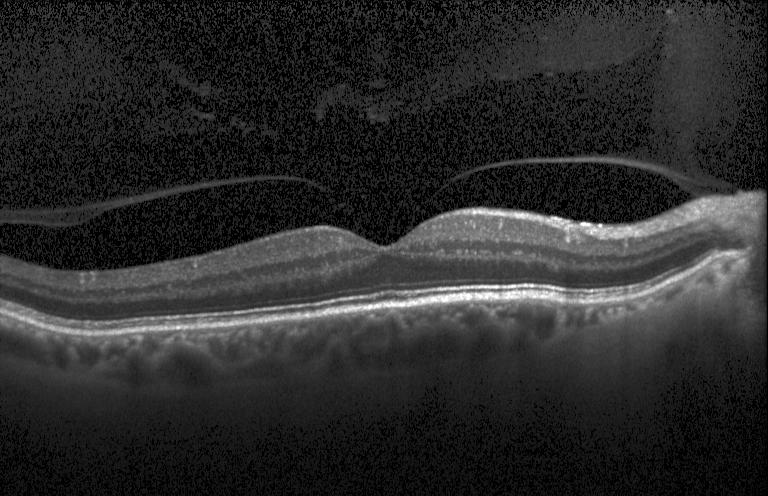 Macular OCT: no evidence of choroidal neovascularization, diabetic macular edema, or drusen.